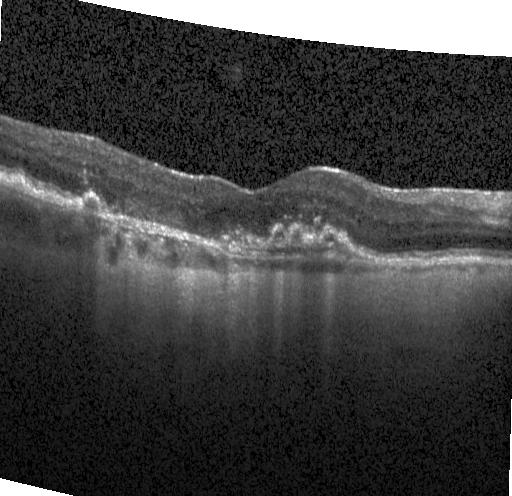

Macular OCT demonstrating CNV.